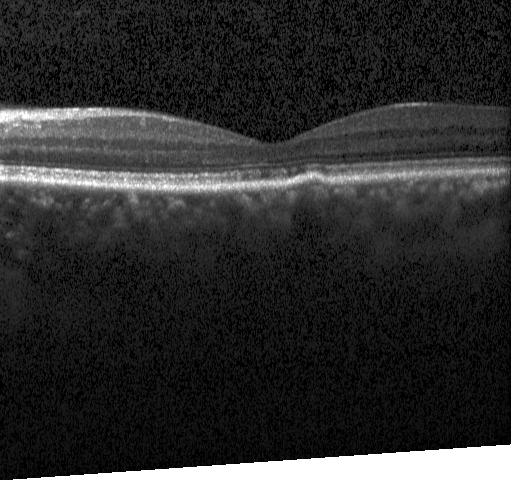
Diagnosis: no evidence of CNV, DME, or drusen.